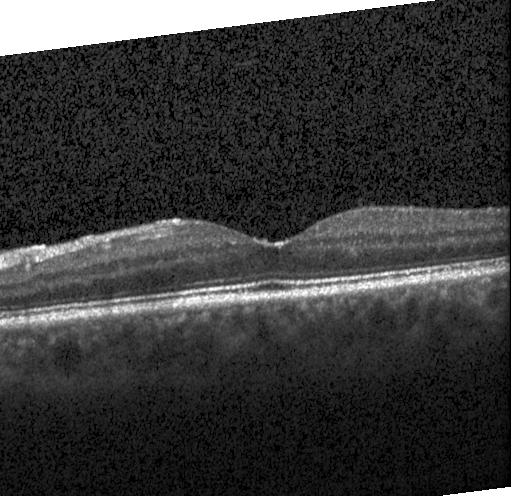
Retinal OCT B-scan · centered on the fovea · acquired on a Heidelberg Spectralis — Impression: neither CNV, DME, nor drusen.